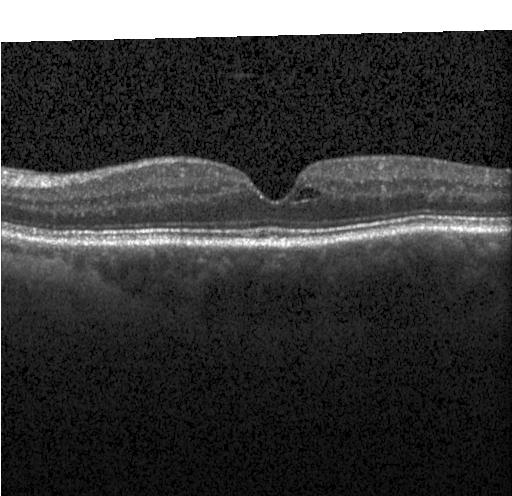
Retinal OCT cross-section showing diabetic macular edema.